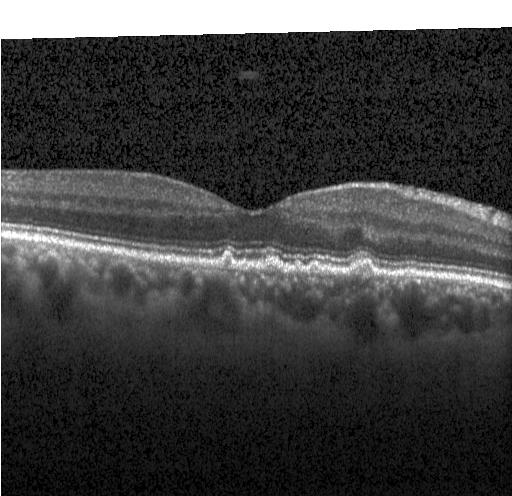

Dx: sub-RPE drusenoid deposits.